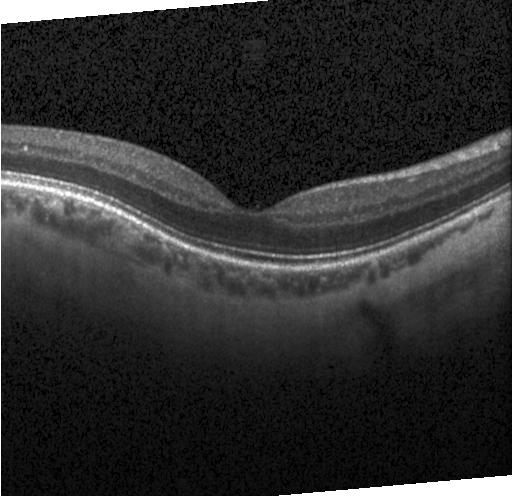
Retinal OCT B-scan. Spectral-domain optical coherence tomography.
Impression: no choroidal neovascularization, no diabetic macular edema, and no drusen.